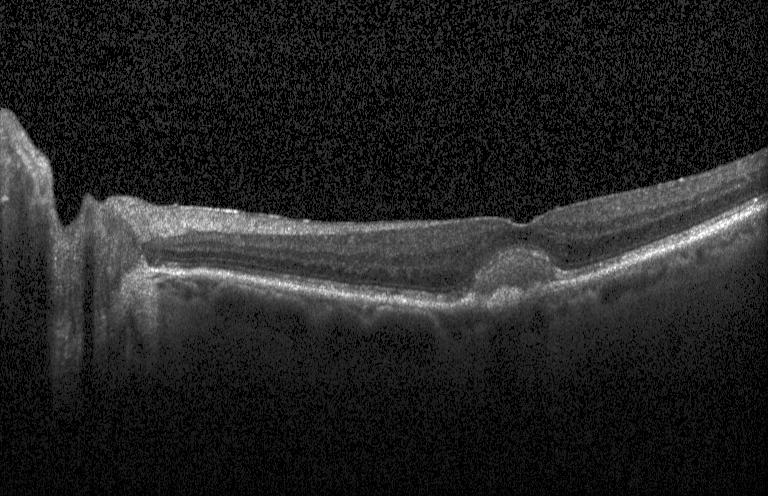 Instrument: Heidelberg Spectralis. OCT B-scan — Assessment: CNV.